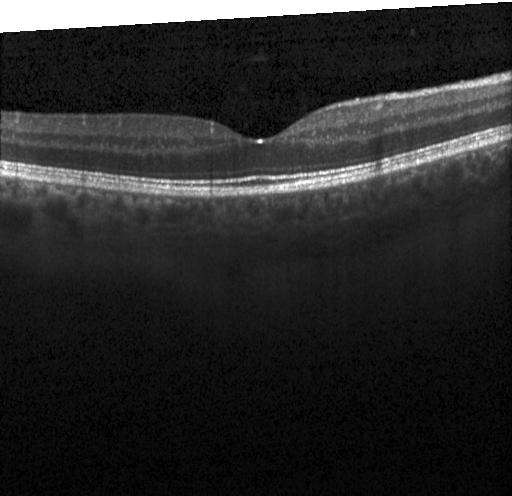
Fovea-centered; acquired on a Heidelberg Spectralis; OCT line scan — Dx: neither choroidal neovascularization, diabetic macular edema, nor drusen.